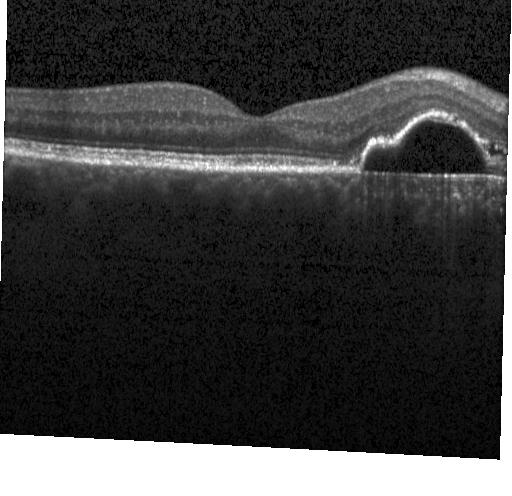 Dx: a choroidal neovascular membrane.